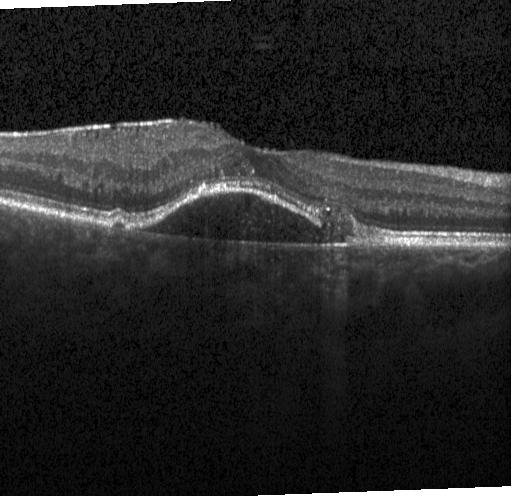

Centered on the fovea; spectral-domain optical coherence tomography; optical coherence tomography scan.
Diagnosis: CNV.